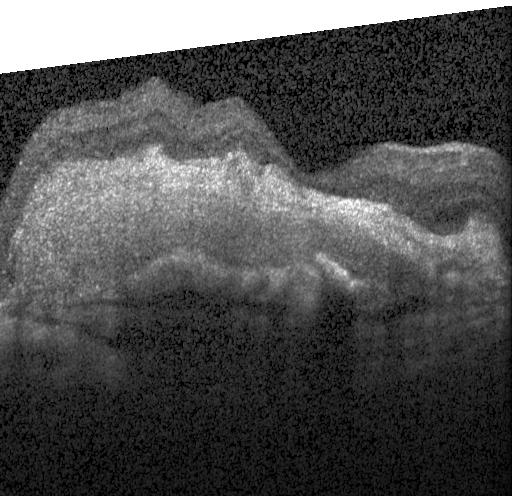 Horizontal scan through the fovea, retinal OCT cross-section. OCT finding: CNV.